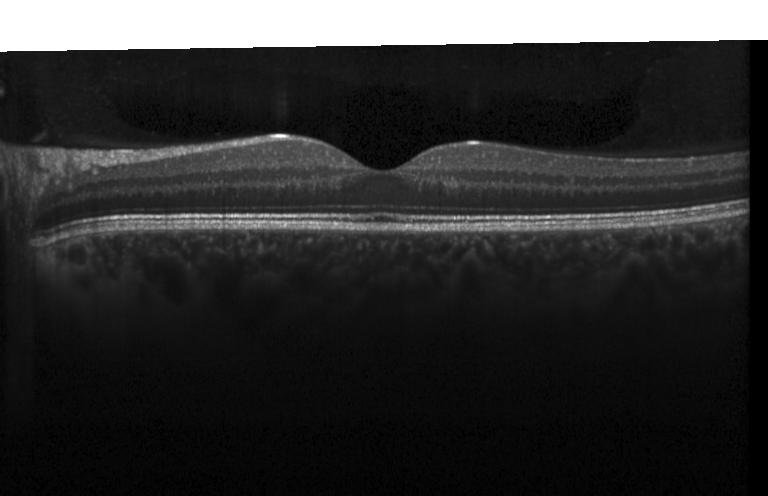
Diagnosis: no evidence of choroidal neovascularization, diabetic macular edema, or drusen.